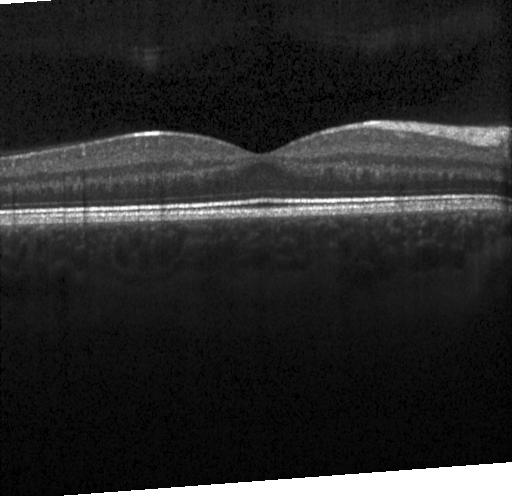

No choroidal neovascularization, diabetic macular edema, or drusen.